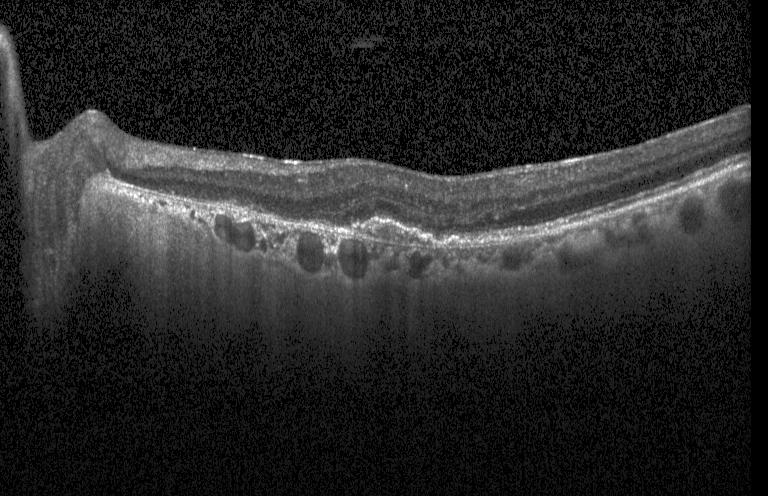
Spectral-domain OCT, optical coherence tomography B-scan, Heidelberg Spectralis — OCT finding: a choroidal neovascular membrane.